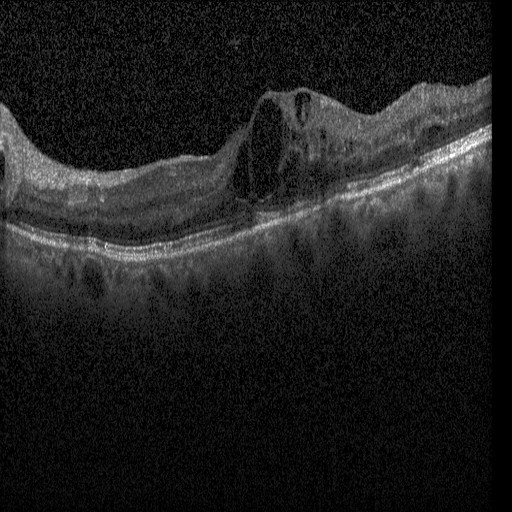

OCT finding: DME.